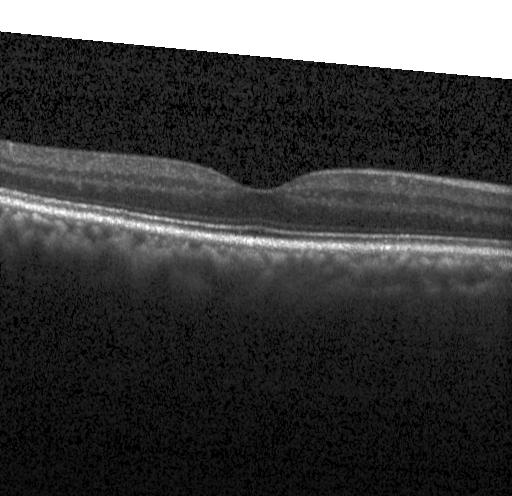
Assessment: neither choroidal neovascularization, diabetic macular edema, nor drusen.